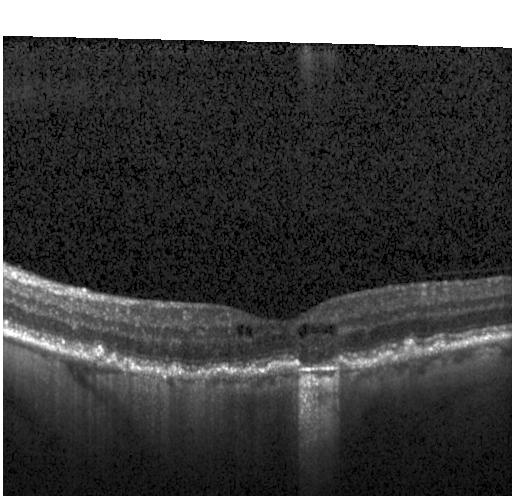

Spectral-domain OCT · instrument: Heidelberg Spectralis · OCT B-scan — Assessment: a choroidal neovascular membrane.